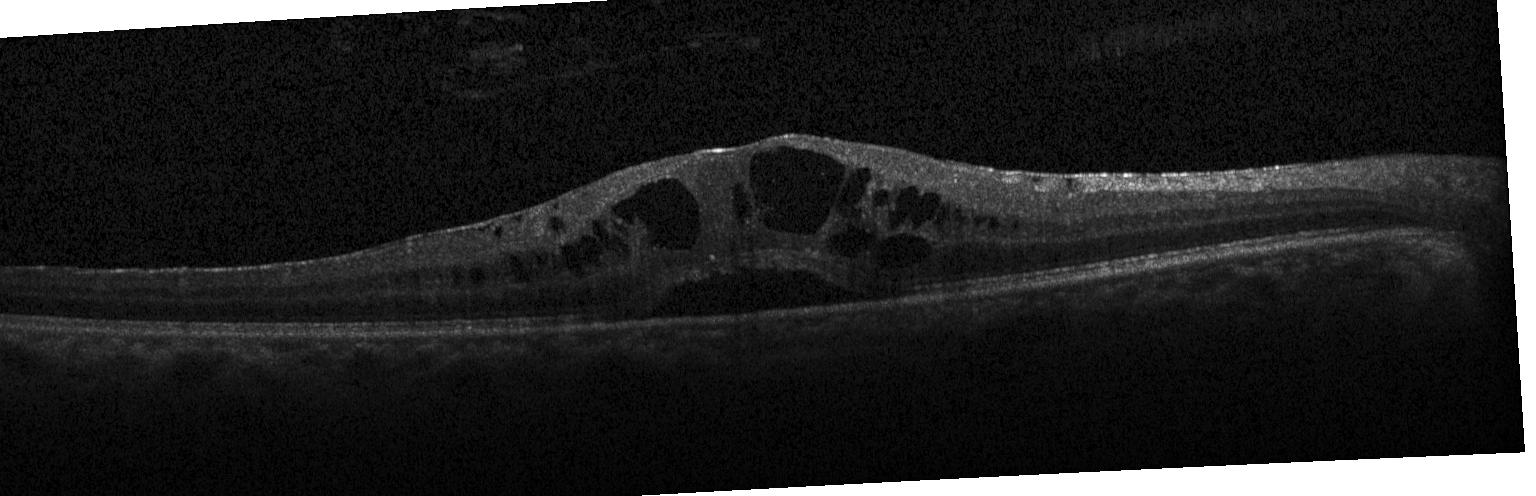
Diagnosis: DME.